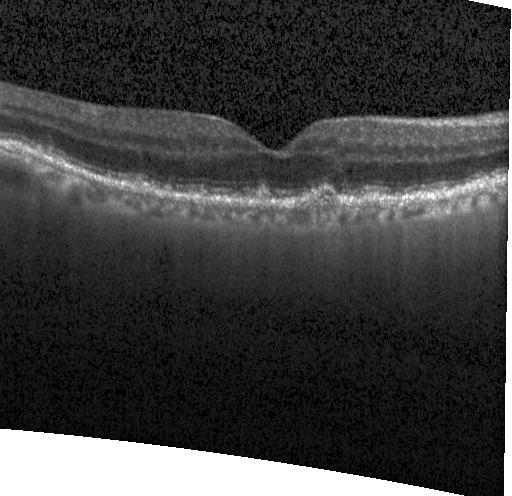

SD-OCT; Heidelberg Spectralis; OCT B-scan; centered on the fovea.
The scan shows drusen.